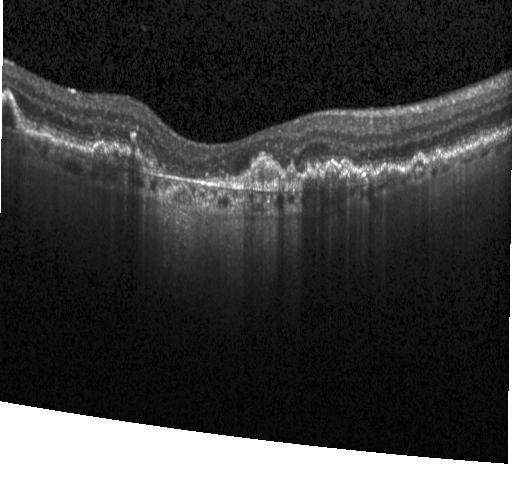

Impression: a choroidal neovascular membrane.